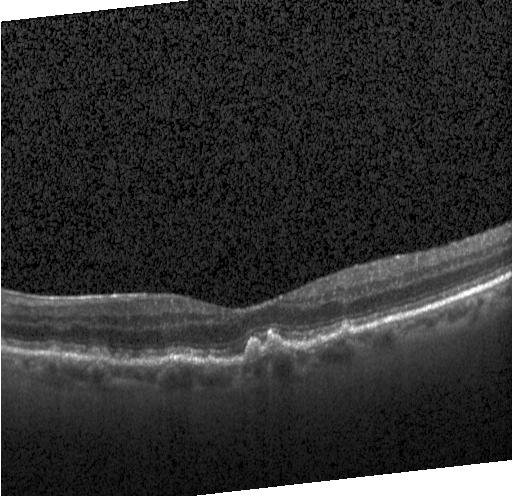

Assessment: sub-RPE drusenoid deposits.